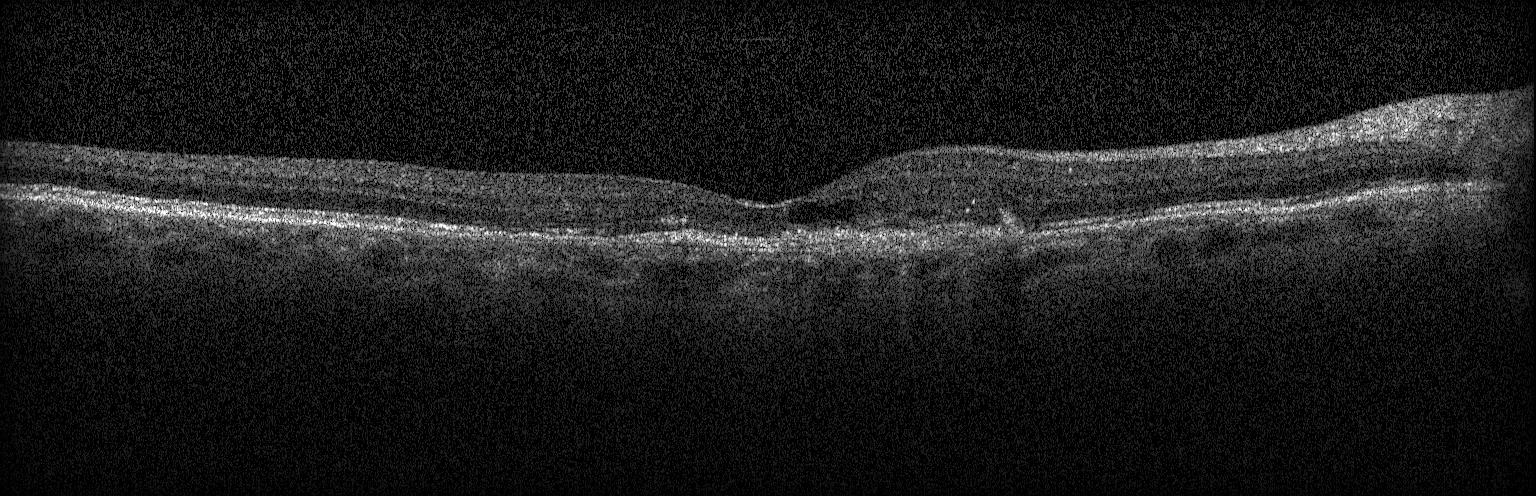

OCT finding: a choroidal neovascular membrane.